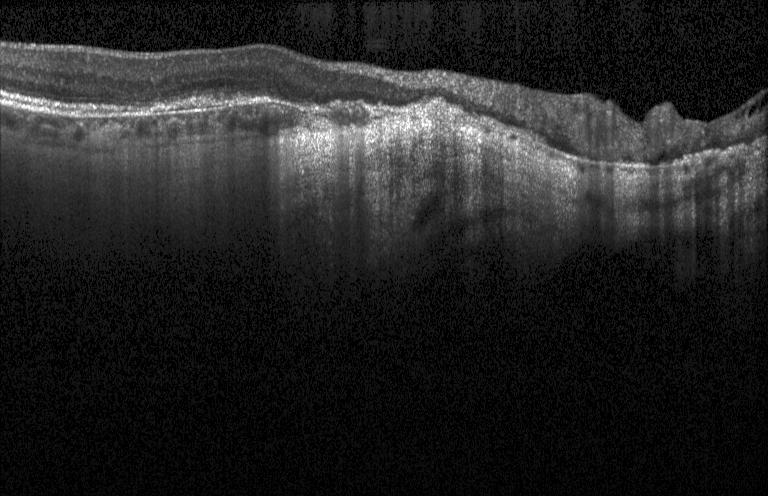
OCT line scan; instrument: Heidelberg Spectralis
The scan shows a choroidal neovascular membrane.